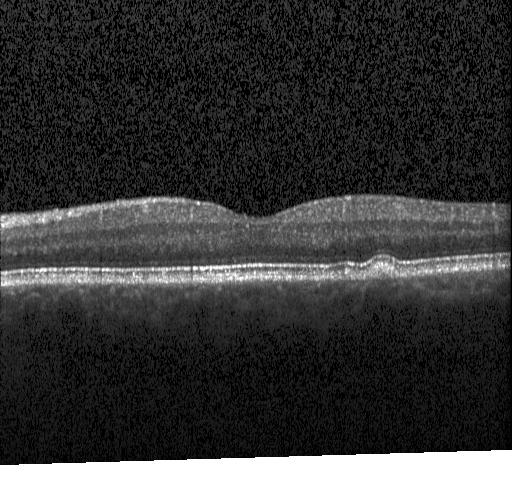
OCT B-scan; spectral-domain OCT
Diagnosis: multiple drusen.